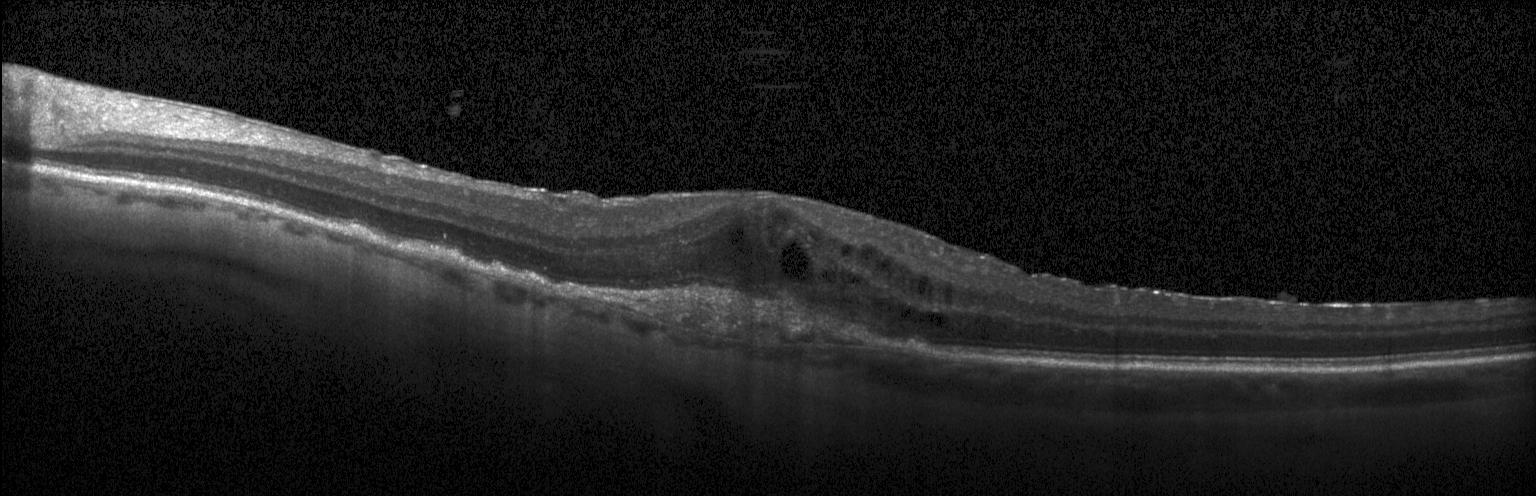 OCT B-scan, centered on the fovea. This B-scan demonstrates a choroidal neovascular membrane.